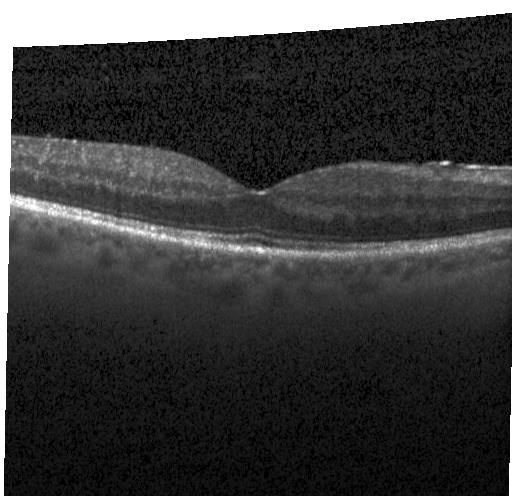
Heidelberg Spectralis OCT system. Through the macula. OCT B-scan
Impression: no CNV, no DME, and no drusen.